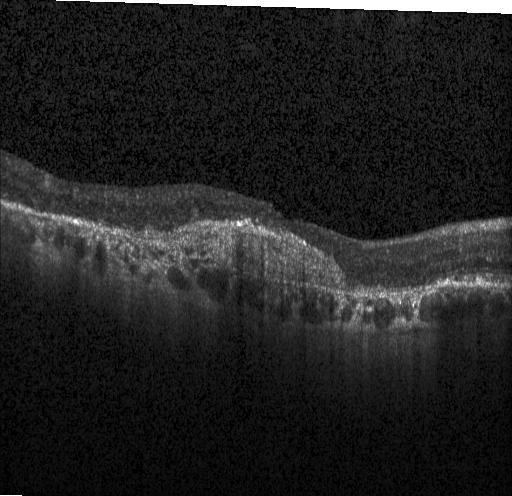

OCT finding: choroidal neovascularization (CNV).